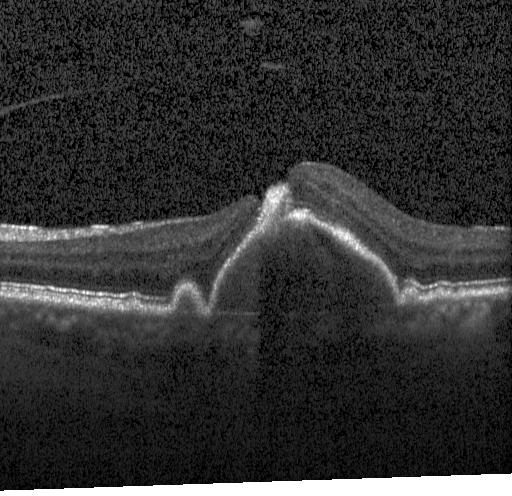
Retinal OCT cross-section, spectral-domain optical coherence tomography, horizontal scan through the fovea. Diagnosis: a choroidal neovascular membrane.